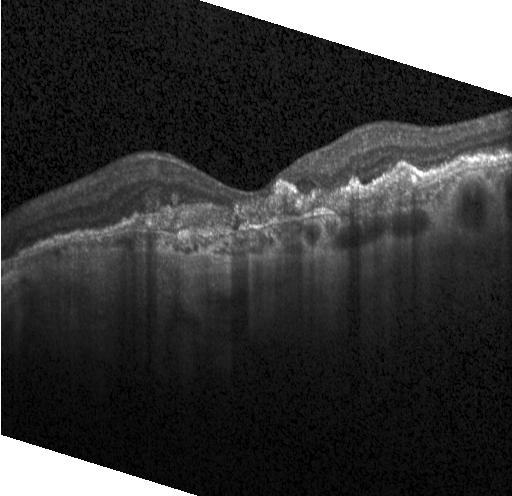 Heidelberg Spectralis · OCT B-scan. Diagnosis: CNV.